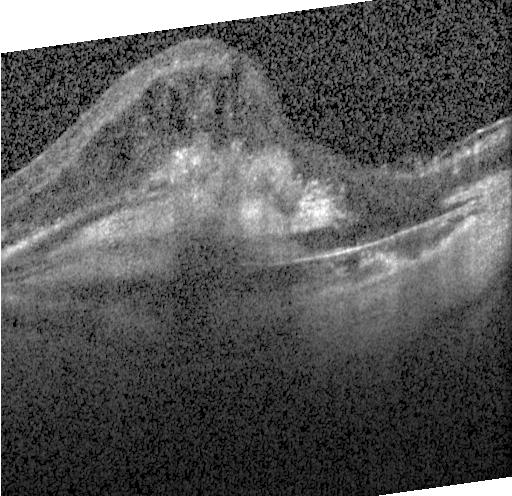 Choroidal neovascularization (CNV).